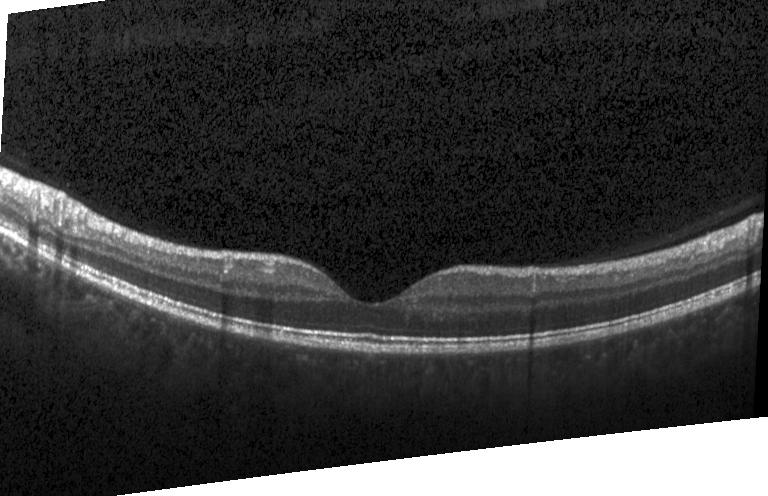
Spectral-domain OCT; retinal OCT cross-section
Diagnosis: no choroidal neovascularization, diabetic macular edema, or drusen.